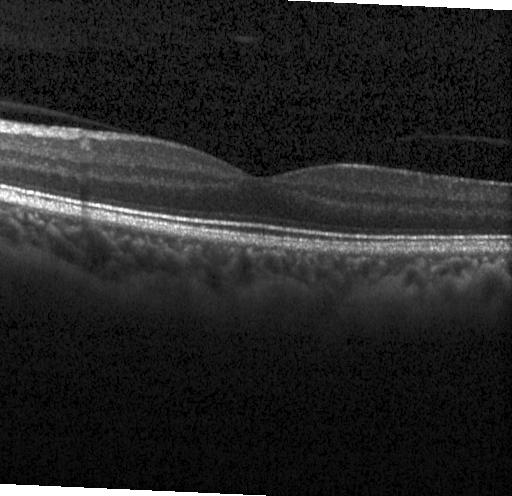
OCT line scan — Assessment: no choroidal neovascularization, diabetic macular edema, or drusen.